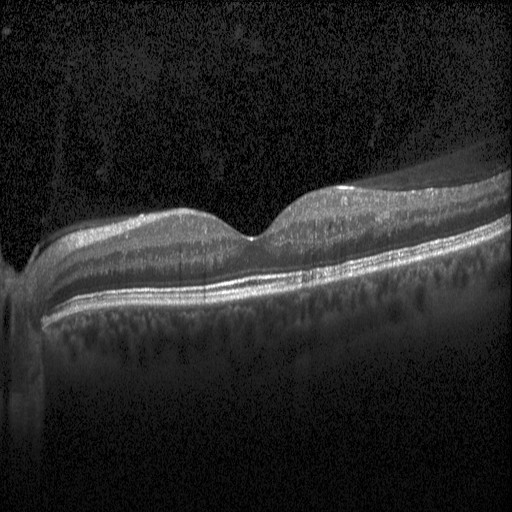

Heidelberg Spectralis; spectral-domain optical coherence tomography; OCT B-scan; fovea-centered. Assessment: DME.